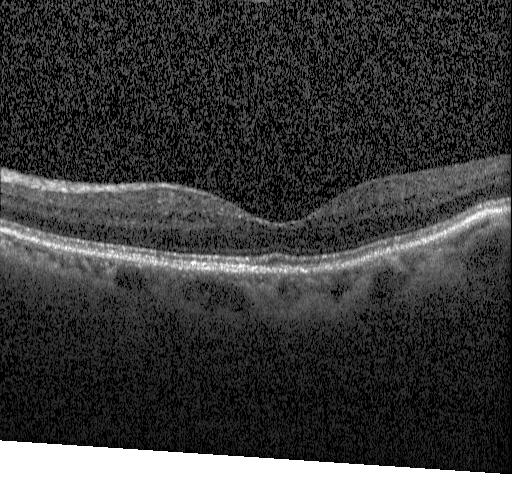 Heidelberg Spectralis · spectral-domain optical coherence tomography · through the macula · OCT line scan.
This B-scan demonstrates no choroidal neovascularization, no diabetic macular edema, and no drusen.